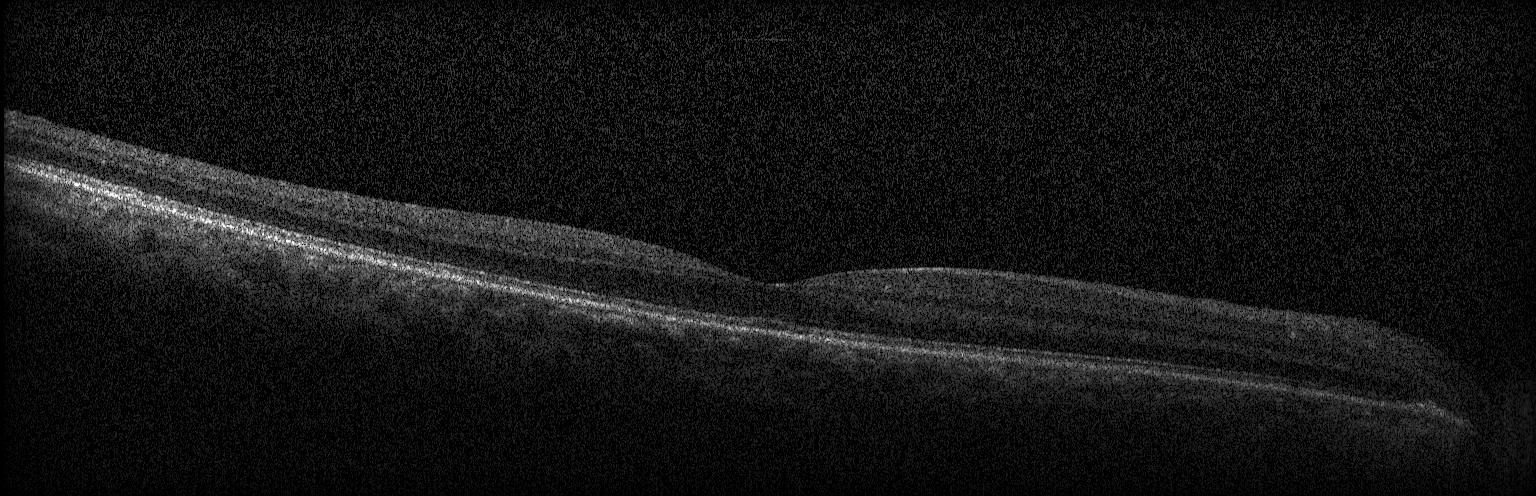

Retinal OCT B-scan. SD-OCT — Finding: no evidence of CNV, DME, or drusen.